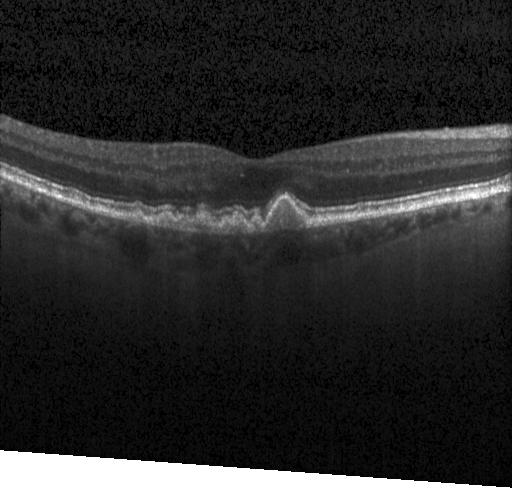

Impression: drusen.